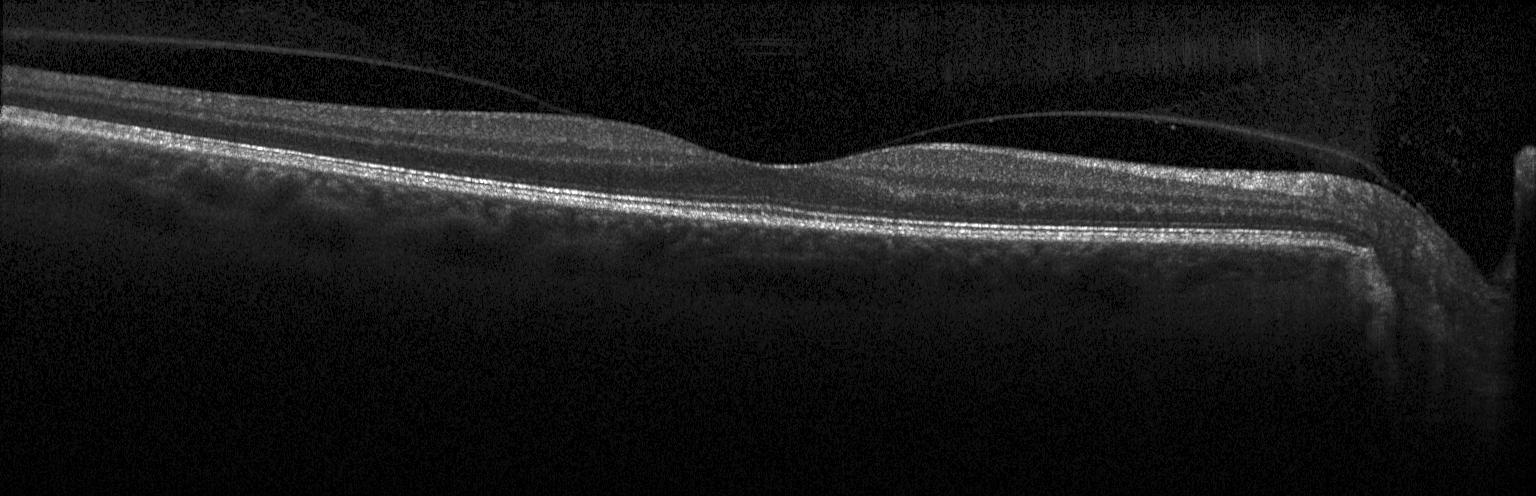 Instrument: Heidelberg Spectralis, retinal OCT B-scan, horizontal scan through the fovea.
Impression: neither choroidal neovascularization, diabetic macular edema, nor drusen.